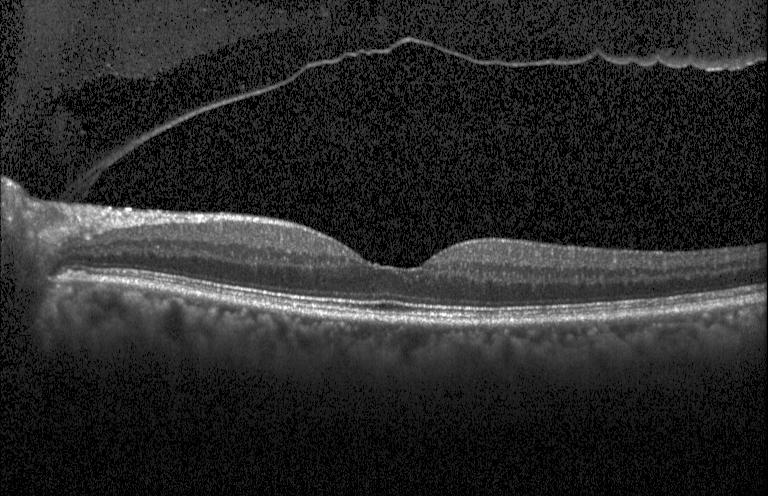
Impression: neither choroidal neovascularization, diabetic macular edema, nor drusen.